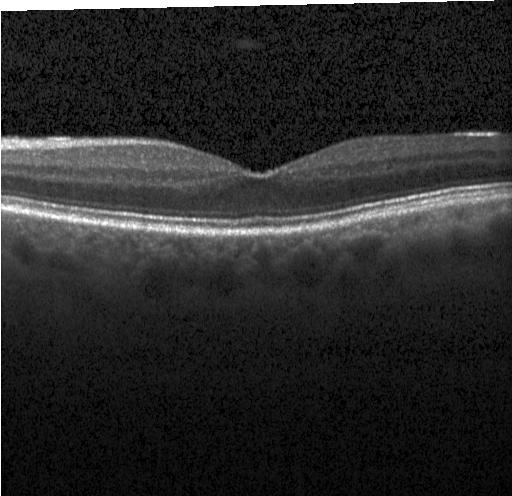 Heidelberg Spectralis, spectral-domain optical coherence tomography, OCT B-scan
The scan shows no choroidal neovascularization, diabetic macular edema, or drusen.